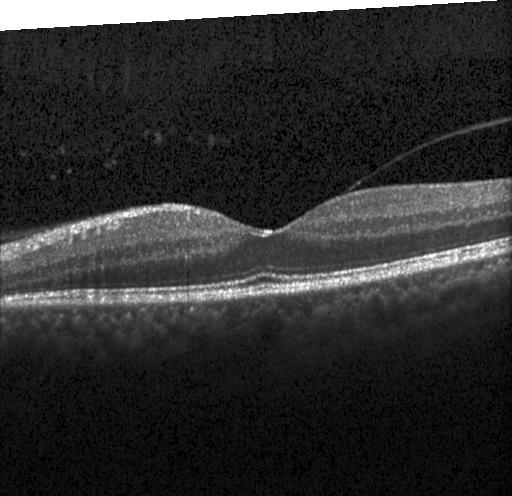

Retinal OCT cross-section showing neither choroidal neovascularization, diabetic macular edema, nor drusen.